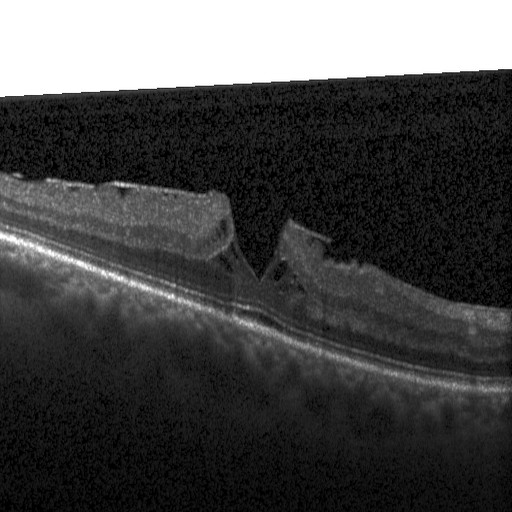
Finding: diabetic macular edema.